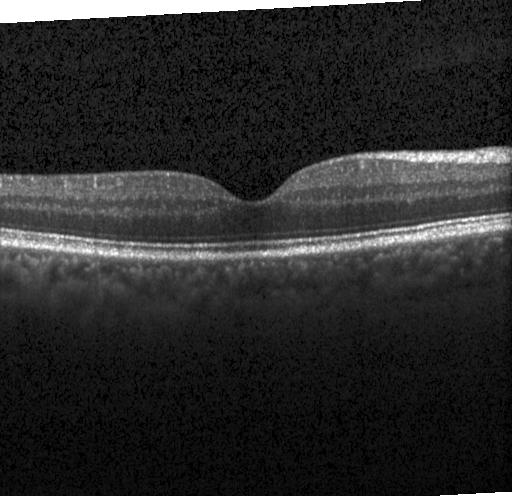 Retinal OCT cross-section. Horizontal scan through the fovea. Spectral-domain optical coherence tomography. Instrument: Heidelberg Spectralis — Macular OCT: no evidence of CNV, DME, or drusen.